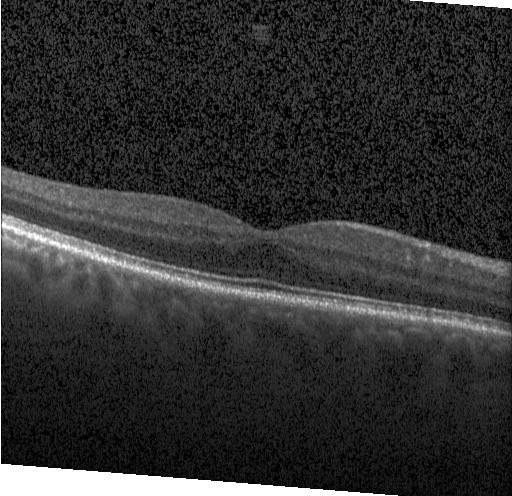
Retinal OCT cross-section showing no choroidal neovascularization, no diabetic macular edema, and no drusen.